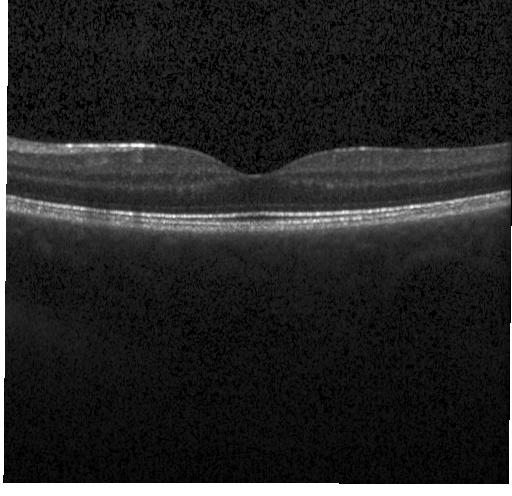
Retinal OCT cross-section · fovea-centered — This B-scan demonstrates neither CNV, DME, nor drusen.